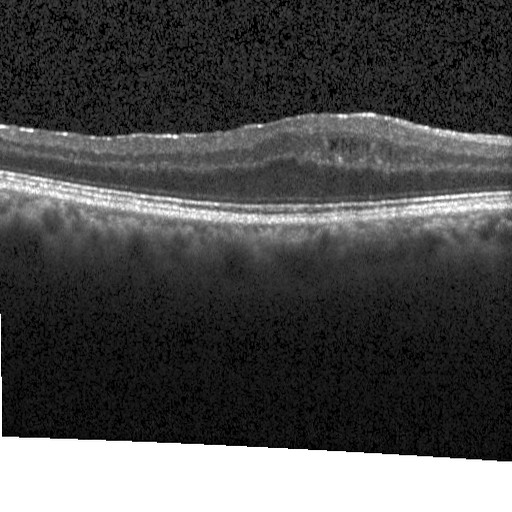

SD-OCT. Horizontal scan through the fovea. OCT B-scan.
Finding: diabetic macular edema (DME).